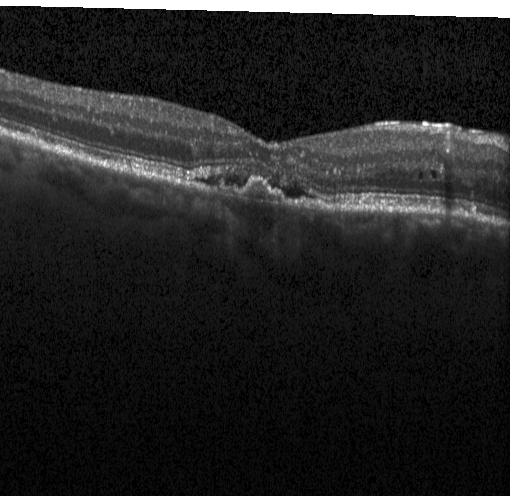
OCT B-scan.
Impression: choroidal neovascularization (CNV).